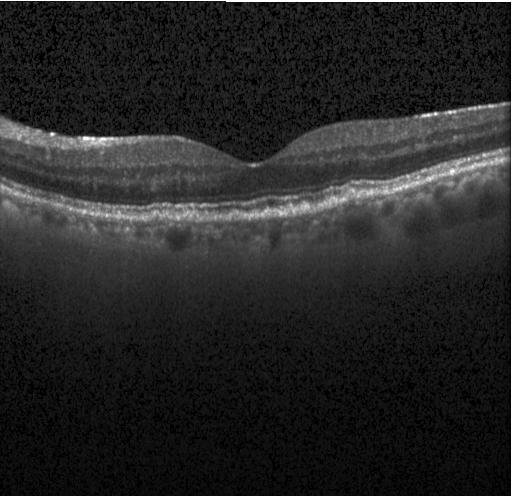 Optical coherence tomography scan — OCT finding: drusen.